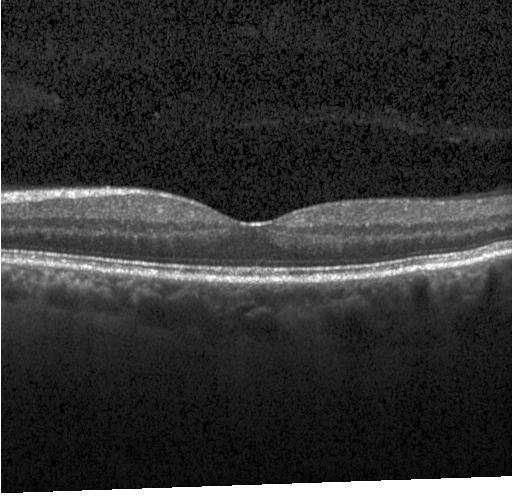

Optical coherence tomography scan — Diagnosis: no CNV, DME, or drusen.